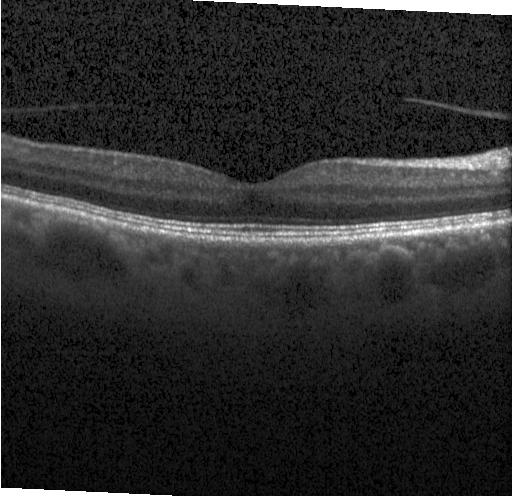 Spectral-domain optical coherence tomography. OCT line scan. Acquired on a Heidelberg Spectralis. Macular scan.
Diagnosis: no choroidal neovascularization, no diabetic macular edema, and no drusen.